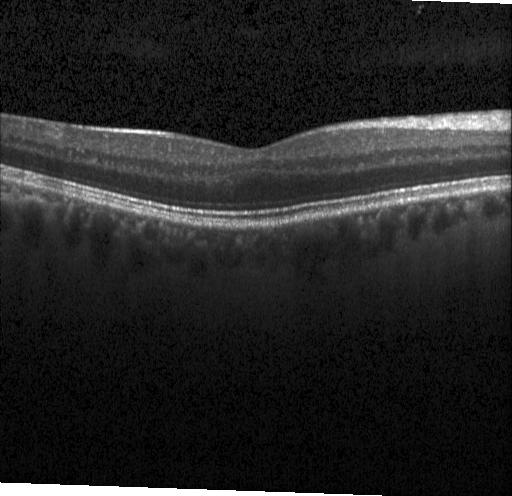

OCT finding: no choroidal neovascularization, no diabetic macular edema, and no drusen.